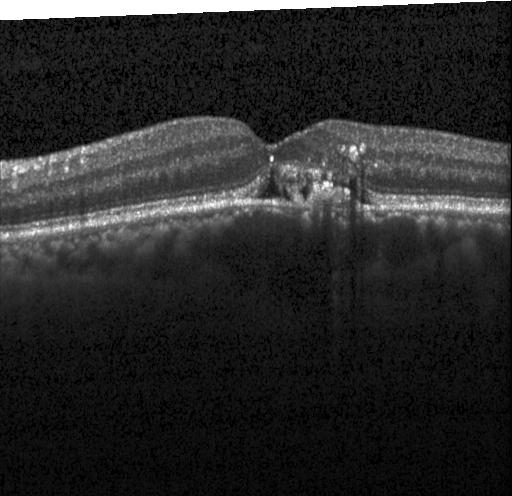
Diagnosis: choroidal neovascularization (CNV).